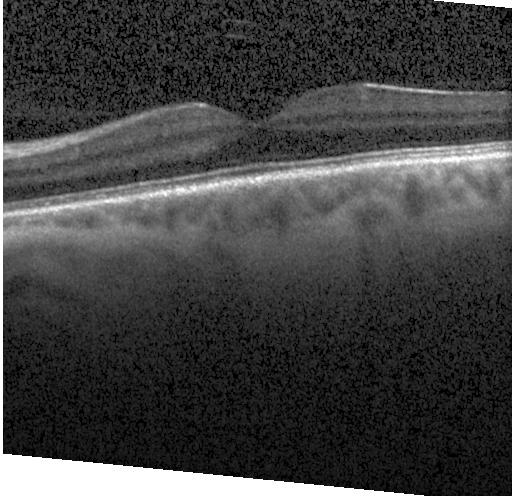 Spectral-domain OCT · macular scan · instrument: Heidelberg Spectralis · OCT line scan. Dx: no choroidal neovascularization, no diabetic macular edema, and no drusen.